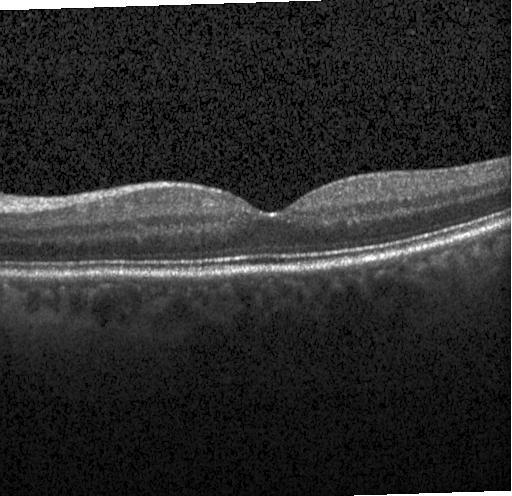

Spectral-domain optical coherence tomography · through the macula · optical coherence tomography scan · Heidelberg Spectralis.
Impression: no choroidal neovascularization, diabetic macular edema, or drusen.